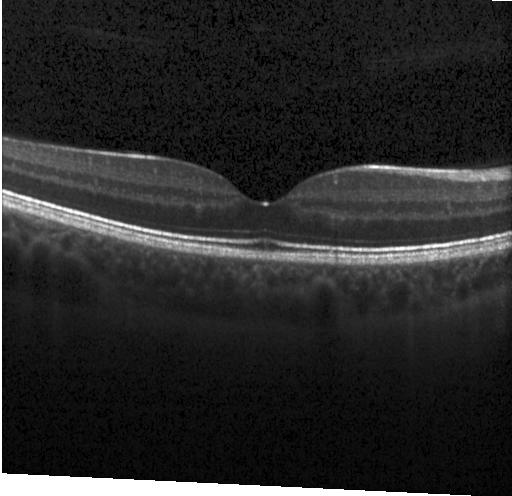

Heidelberg Spectralis, spectral-domain OCT, OCT line scan, through the macula. Impression: no choroidal neovascularization, no diabetic macular edema, and no drusen.